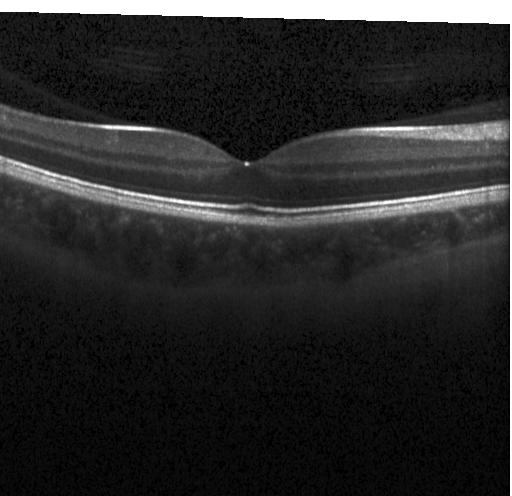 Heidelberg Spectralis OCT system; optical coherence tomography scan; spectral-domain optical coherence tomography; fovea-centered
Diagnosis: no evidence of choroidal neovascularization, diabetic macular edema, or drusen.